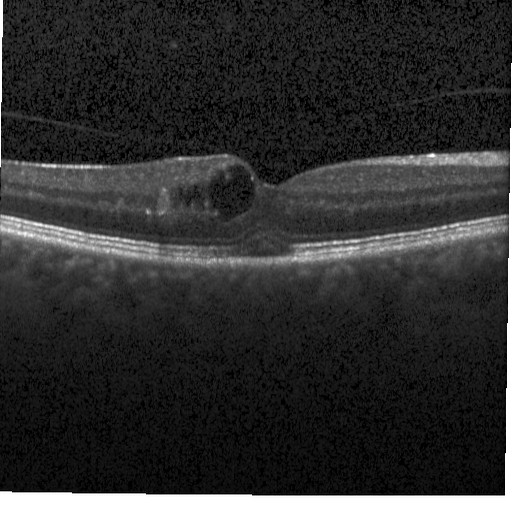

Finding: diabetic macular edema.